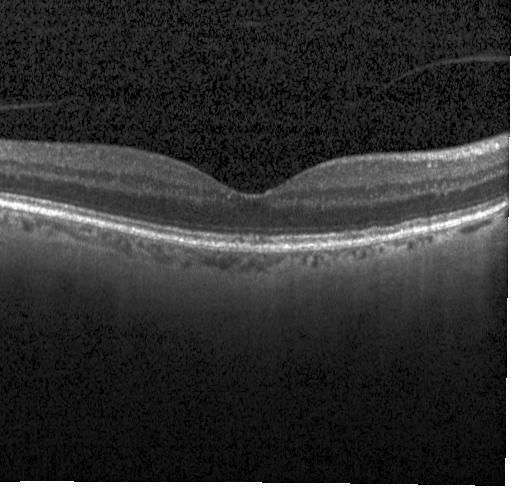

Impression: no choroidal neovascularization, diabetic macular edema, or drusen.